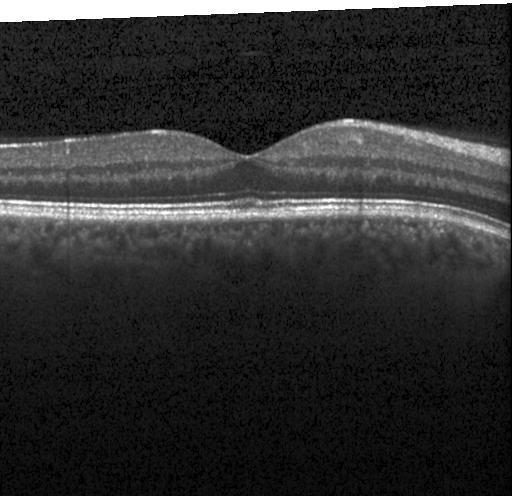

SD-OCT; retinal OCT B-scan. The scan shows no choroidal neovascularization, no diabetic macular edema, and no drusen.